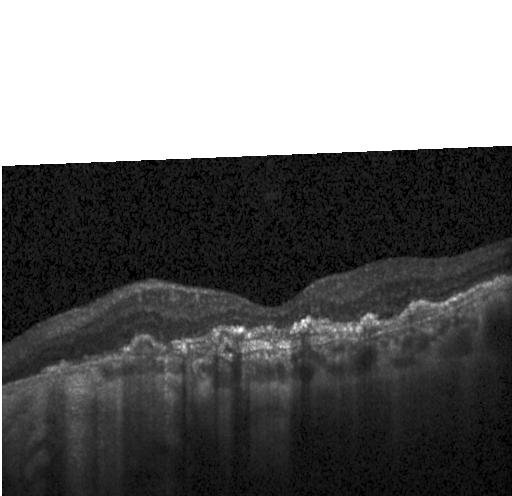

Optical coherence tomography B-scan; spectral-domain OCT; Heidelberg Spectralis. The scan shows choroidal neovascularization (CNV).